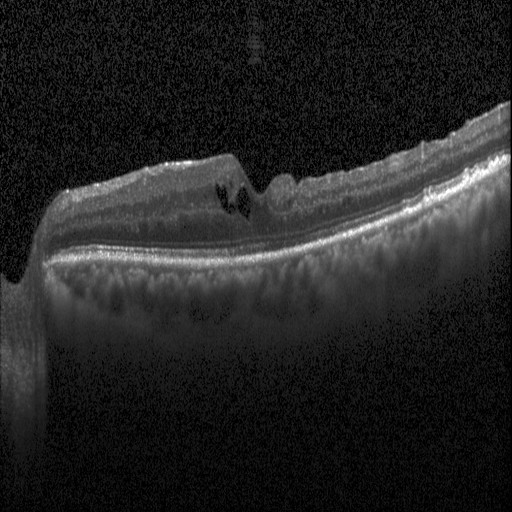 Retinal OCT cross-section, Heidelberg Spectralis, through the macula, spectral-domain optical coherence tomography. Diagnosis: diabetic macular edema (DME).